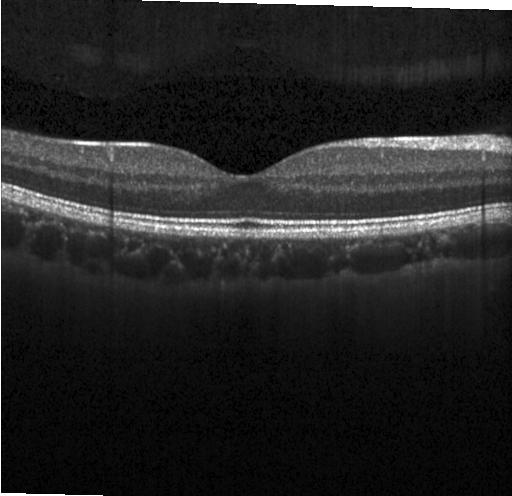 Macular scan; spectral-domain OCT; retinal OCT cross-section. Assessment: neither choroidal neovascularization, diabetic macular edema, nor drusen.